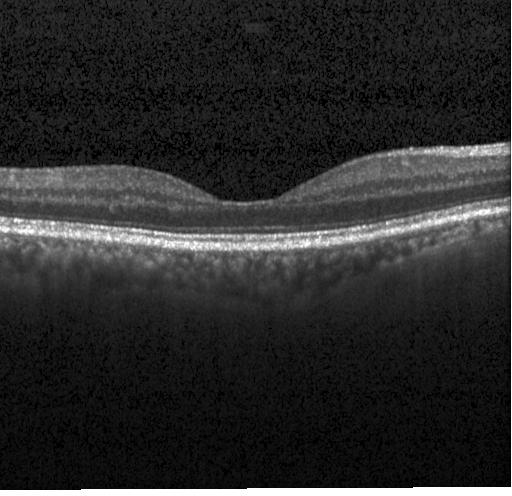
Macular OCT: no CNV, no DME, and no drusen.